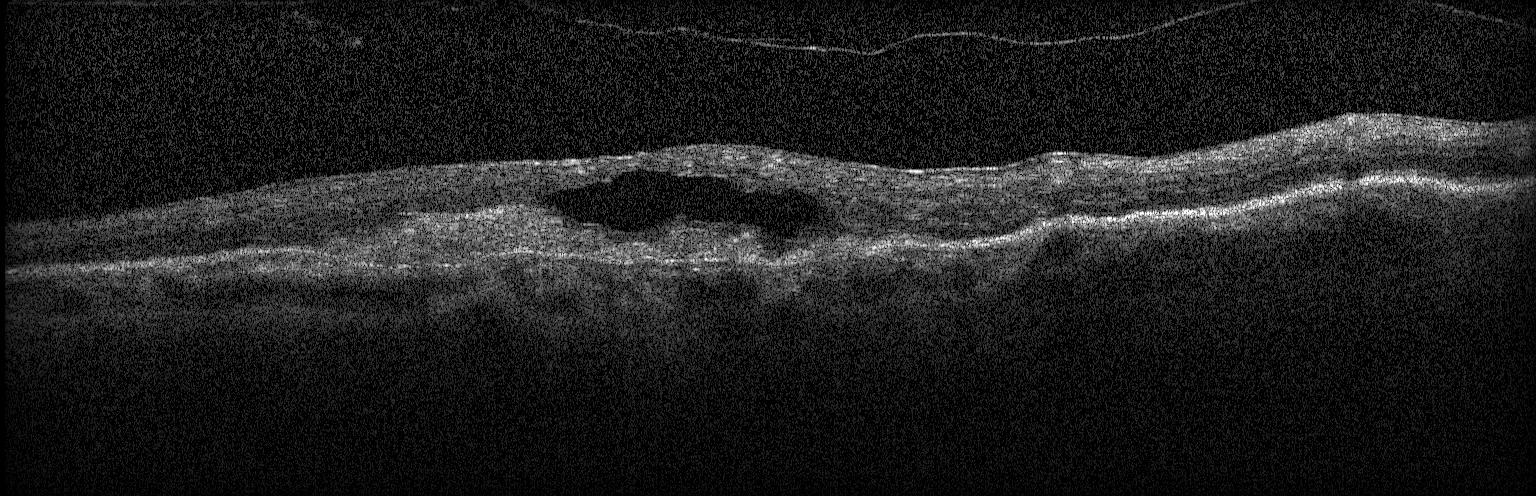

Diagnosis: a choroidal neovascular membrane.